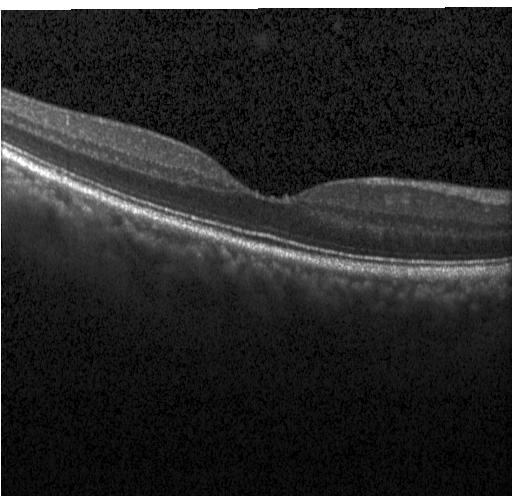 OCT B-scan. Horizontal scan through the fovea.
Macular OCT: neither choroidal neovascularization, diabetic macular edema, nor drusen.